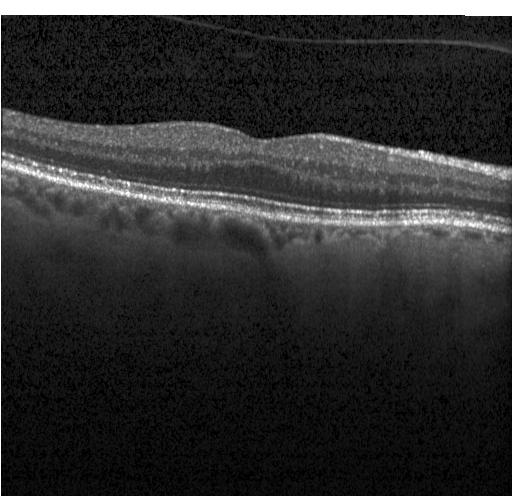 Optical coherence tomography scan
Macular OCT: no choroidal neovascularization, diabetic macular edema, or drusen.